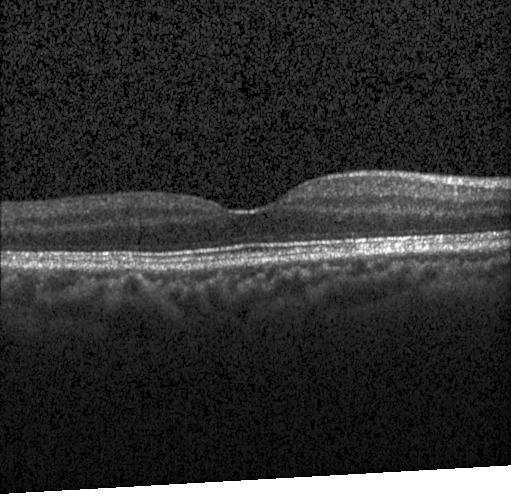

Horizontal scan through the fovea. OCT line scan.
Finding: no CNV, DME, or drusen.